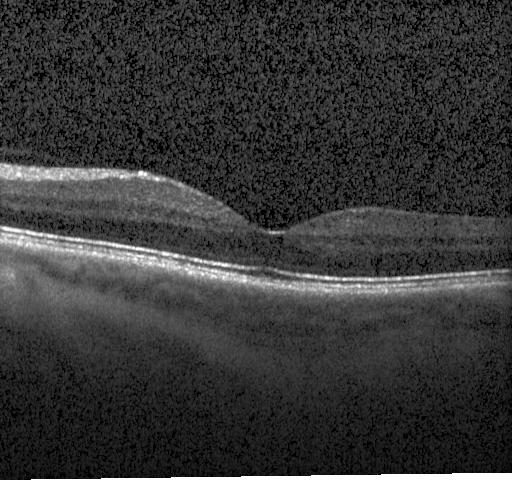
OCT finding: no CNV, no DME, and no drusen.